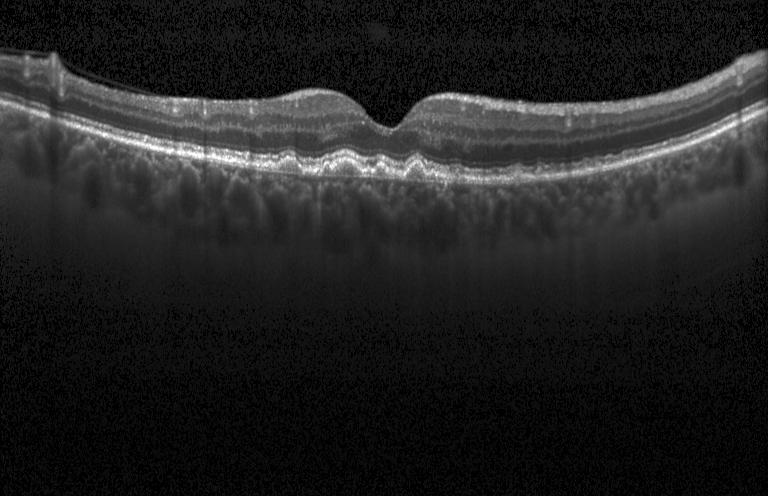

Retinal OCT cross-section. SD-OCT. Centered on the fovea. Heidelberg Spectralis OCT system.
Macular OCT: drusen.